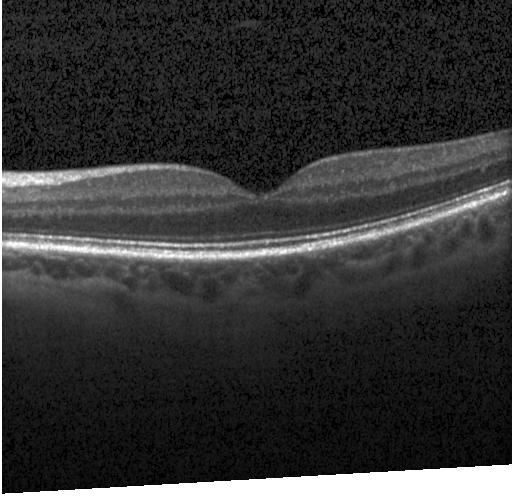 OCT line scan. Spectral-domain OCT.
Dx: no choroidal neovascularization, no diabetic macular edema, and no drusen.